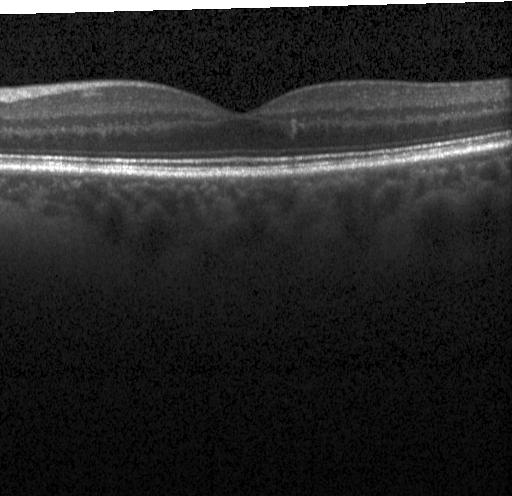
Impression: no choroidal neovascularization, diabetic macular edema, or drusen.